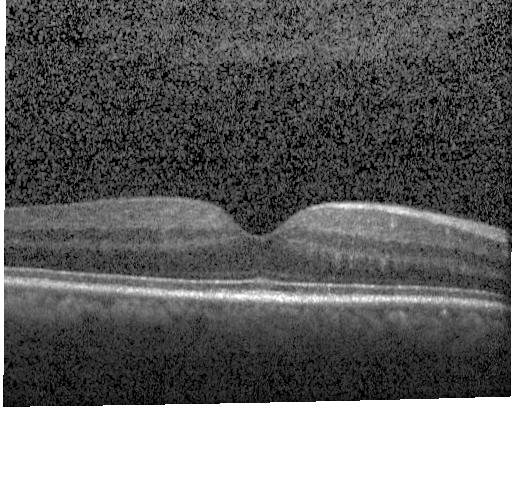
OCT B-scan · SD-OCT — The scan shows no evidence of choroidal neovascularization, diabetic macular edema, or drusen.